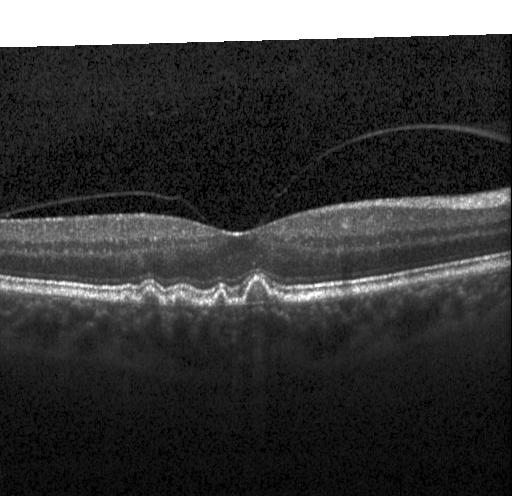

Through the macula; Heidelberg Spectralis OCT system; OCT B-scan
Multiple drusen.